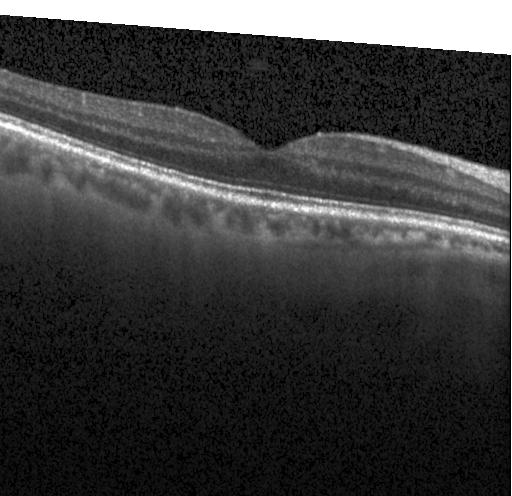 Heidelberg Spectralis; optical coherence tomography scan.
Finding: neither choroidal neovascularization, diabetic macular edema, nor drusen.